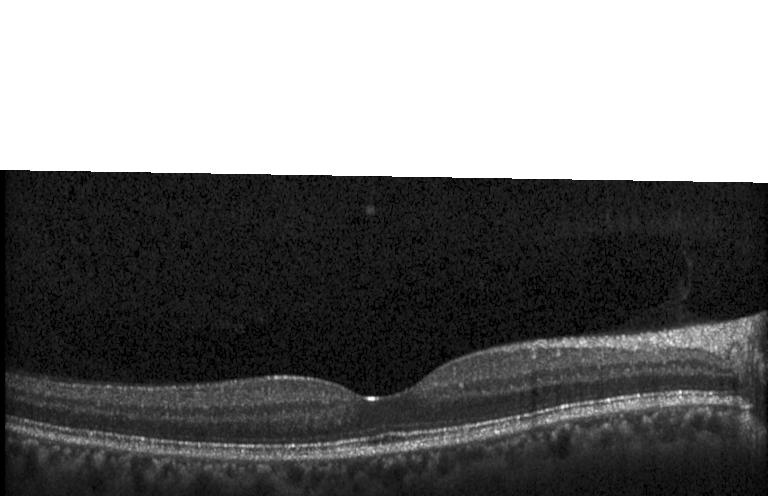 Retinal OCT B-scan. Spectral-domain optical coherence tomography. Macular scan. Instrument: Heidelberg Spectralis
No evidence of choroidal neovascularization, diabetic macular edema, or drusen.